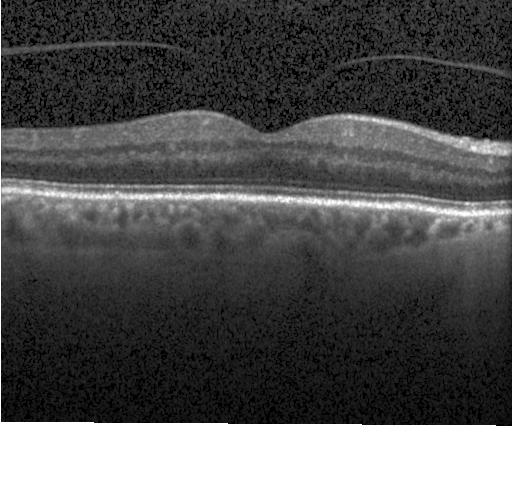

Optical coherence tomography B-scan. Through the macula. SD-OCT. Heidelberg Spectralis — The scan shows no CNV, no DME, and no drusen.